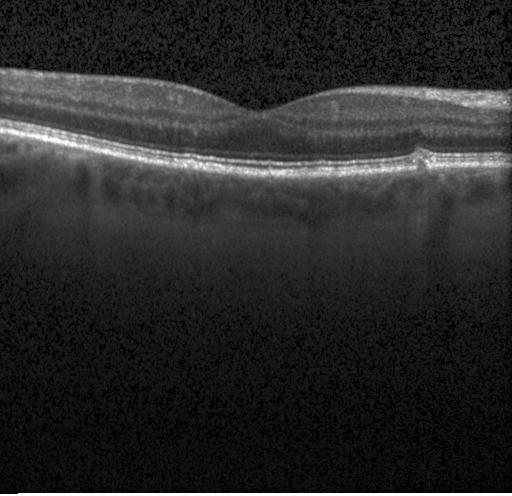

Assessment: drusen.